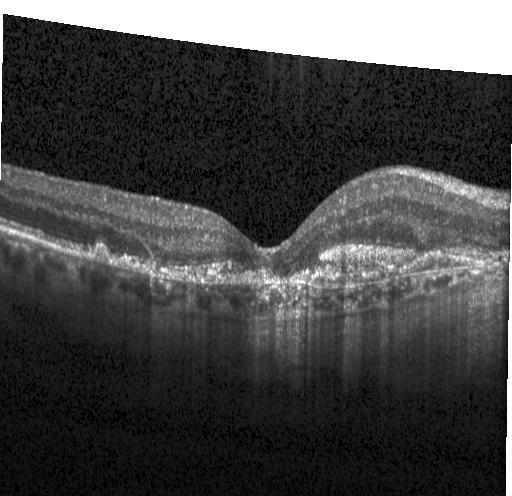 Finding: a choroidal neovascular membrane.